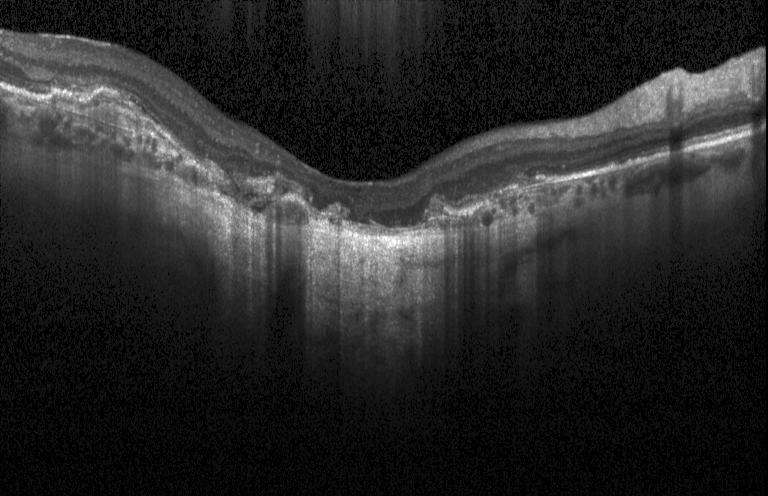 Spectral-domain OCT B-scan: a choroidal neovascular membrane.